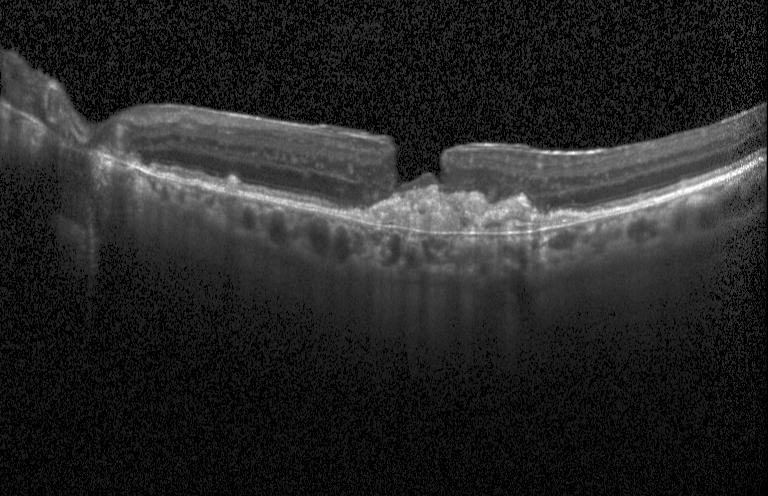

Acquired on a Heidelberg Spectralis · optical coherence tomography B-scan — Macular OCT: a choroidal neovascular membrane.